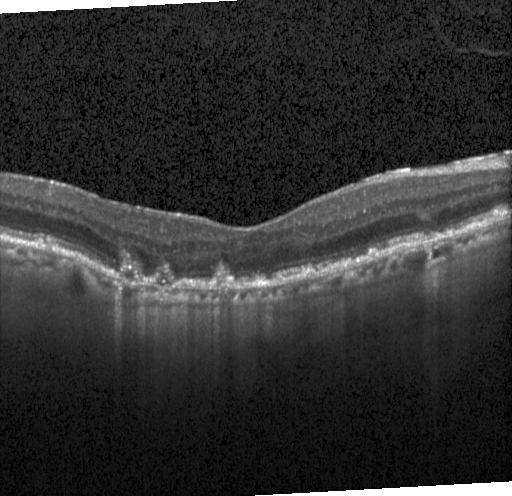
Spectral-domain optical coherence tomography. Optical coherence tomography scan. Fovea-centered. Dx: CNV.